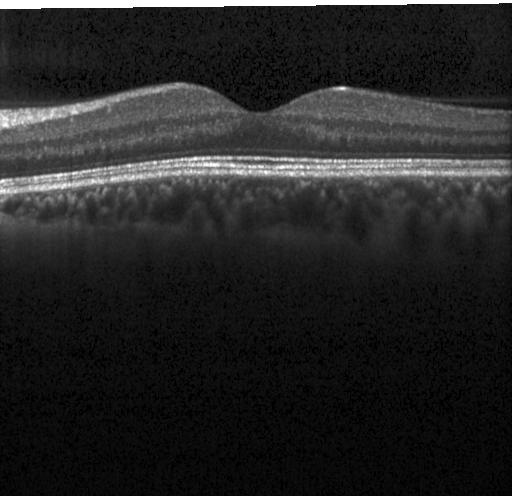 OCT finding: no evidence of CNV, DME, or drusen.